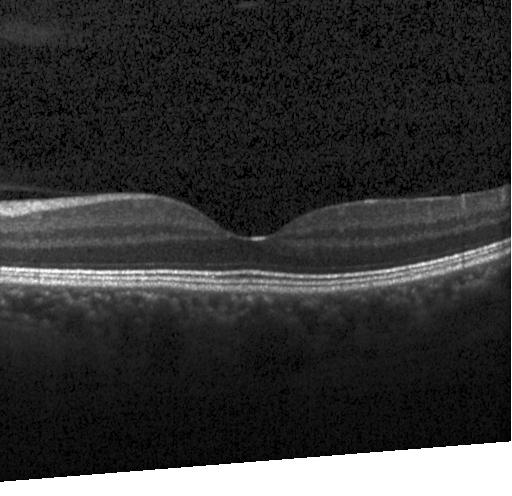

Finding: no evidence of choroidal neovascularization, diabetic macular edema, or drusen.